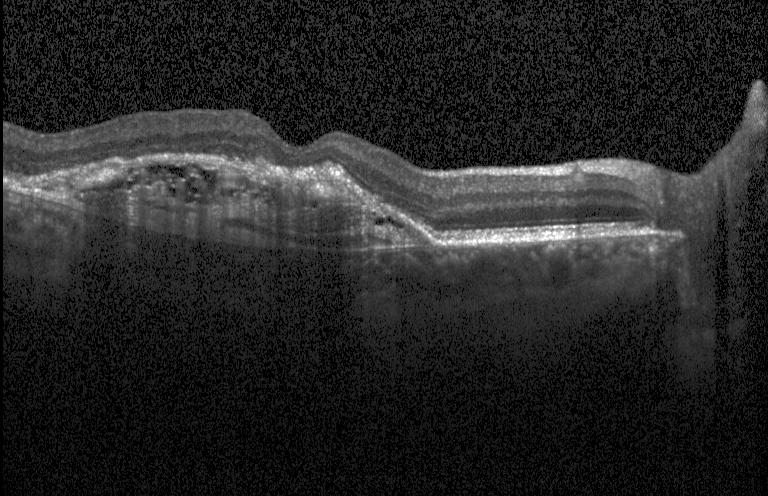 Spectral-domain OCT · retinal OCT B-scan.
Choroidal neovascularization (CNV).